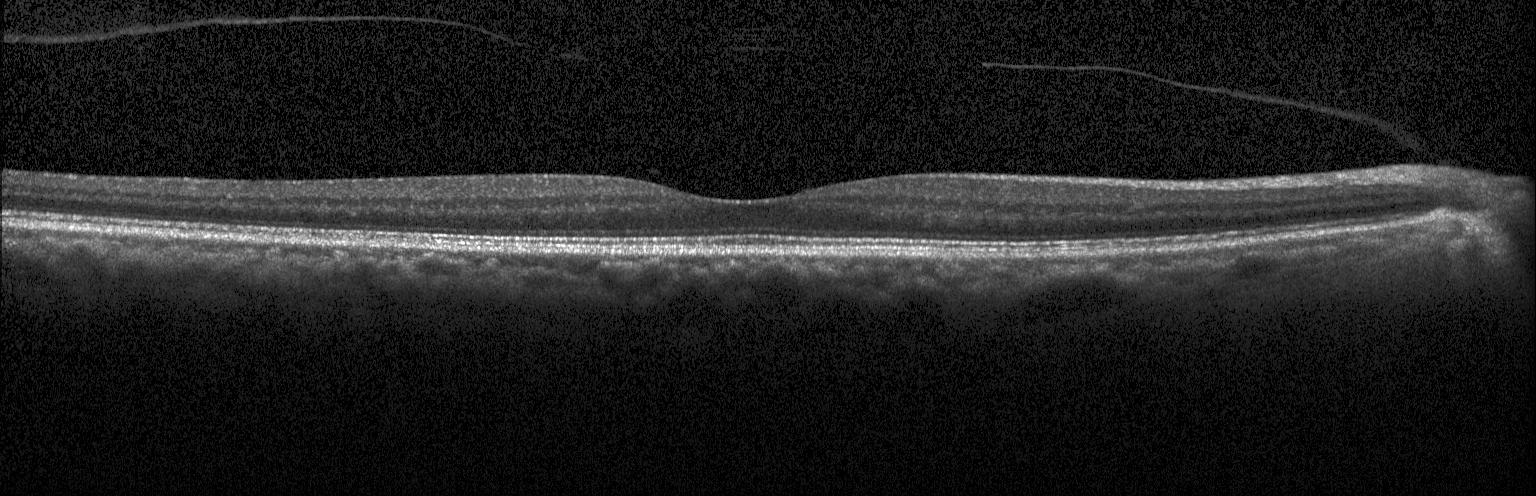 The scan shows no choroidal neovascularization, no diabetic macular edema, and no drusen.